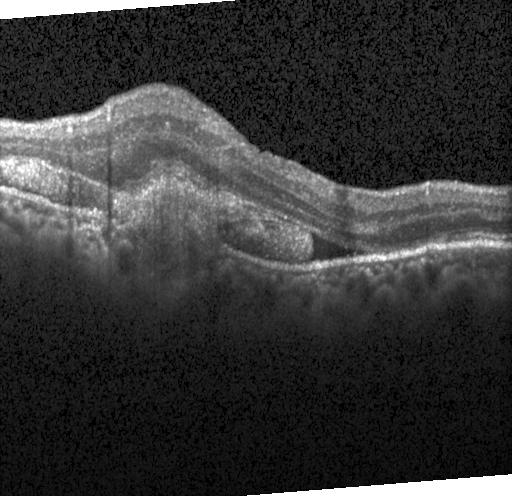

Retinal OCT B-scan, centered on the fovea. Impression: a choroidal neovascular membrane.